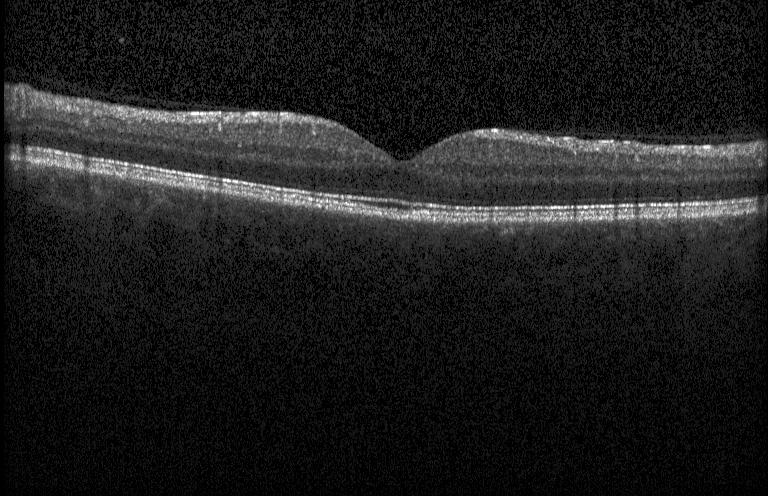
Optical coherence tomography B-scan — Diagnosis: neither choroidal neovascularization, diabetic macular edema, nor drusen.